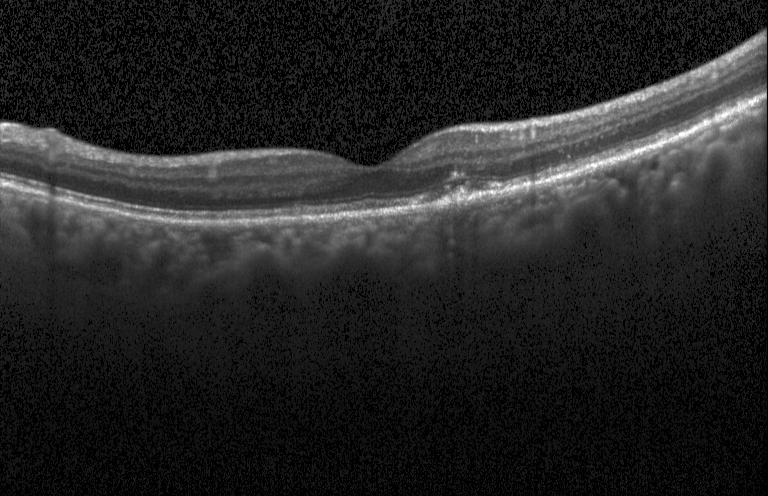

SD-OCT, acquired on a Heidelberg Spectralis, optical coherence tomography scan, centered on the fovea
Diagnosis: sub-RPE drusenoid deposits.